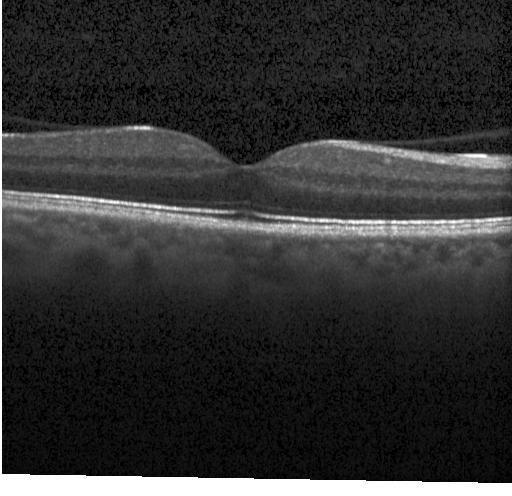

Dx: neither choroidal neovascularization, diabetic macular edema, nor drusen.